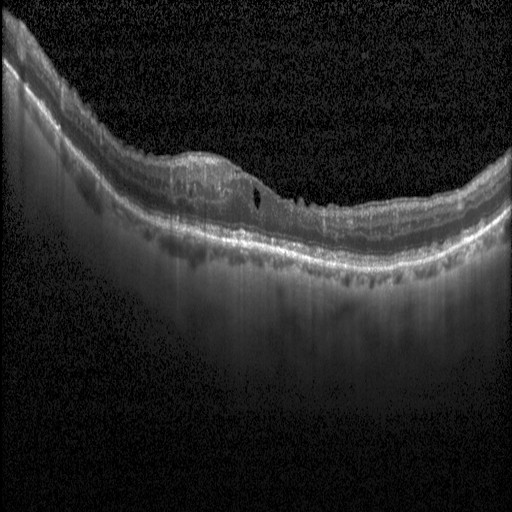
Optical coherence tomography B-scan. SD-OCT. Acquired on a Heidelberg Spectralis. Centered on the fovea. Impression: DME.